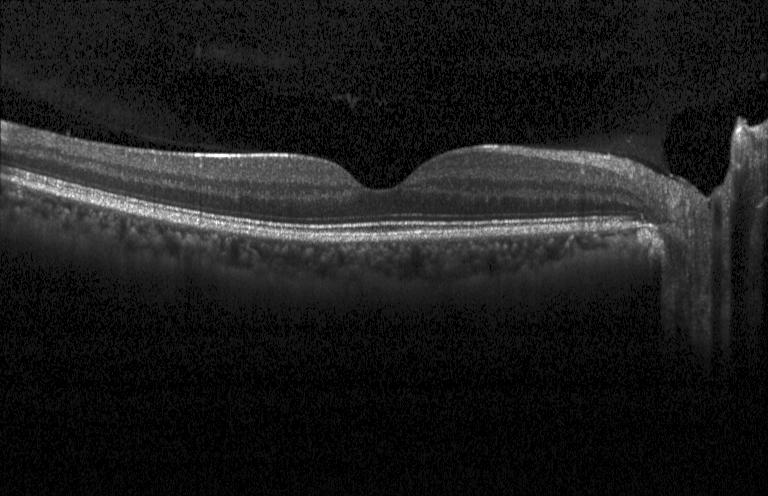 No evidence of choroidal neovascularization, diabetic macular edema, or drusen.